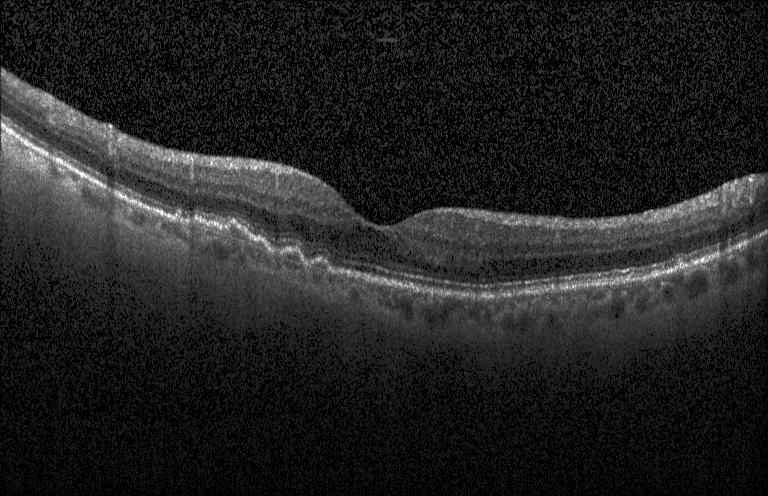

OCT finding: drusen.